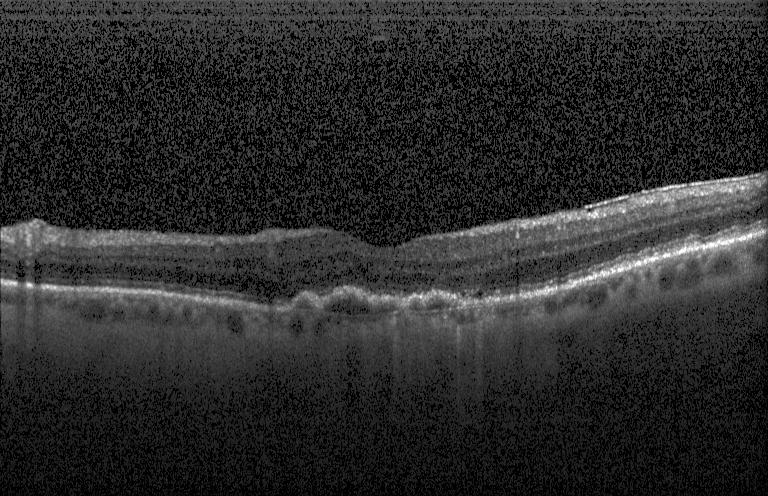

Spectral-domain optical coherence tomography, optical coherence tomography scan. Impression: a choroidal neovascular membrane.